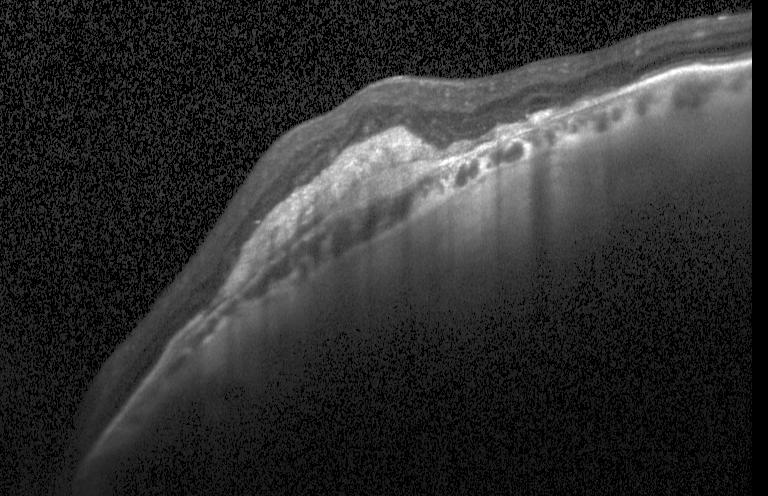

Spectral-domain optical coherence tomography; optical coherence tomography scan; macular scan; acquired on a Heidelberg Spectralis. Diagnosis: choroidal neovascularization (CNV).